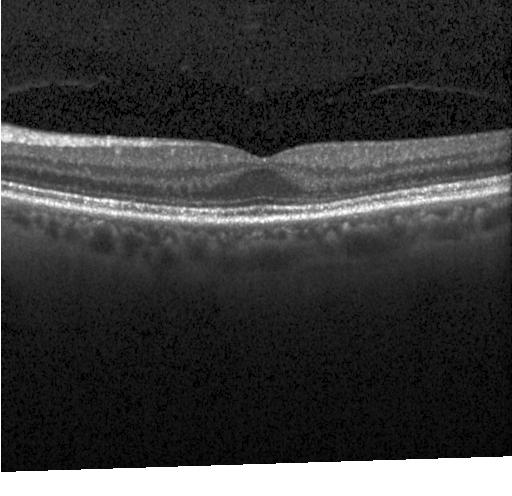
Optical coherence tomography scan · spectral-domain optical coherence tomography.
Neither choroidal neovascularization, diabetic macular edema, nor drusen.